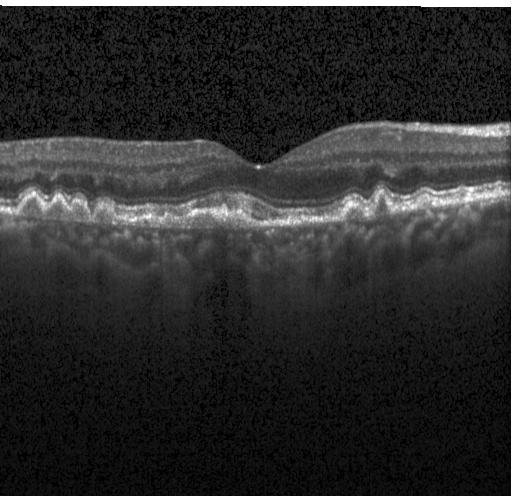

Instrument: Heidelberg Spectralis, spectral-domain OCT, OCT line scan — This B-scan demonstrates multiple drusen.